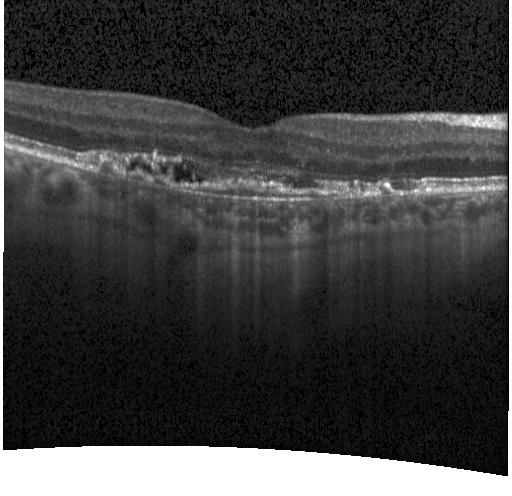
Through the macula. Retinal OCT B-scan
Finding: a choroidal neovascular membrane.